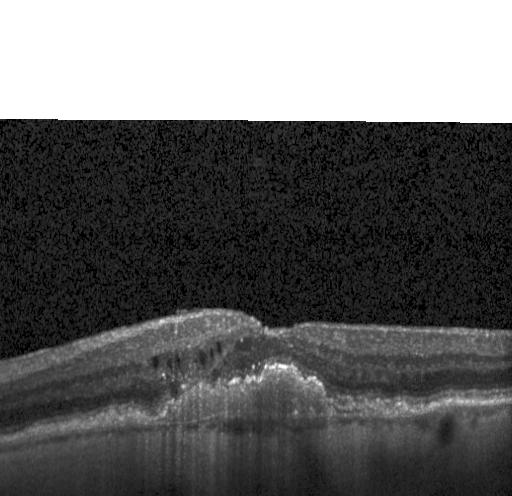

OCT B-scan showing a choroidal neovascular membrane.